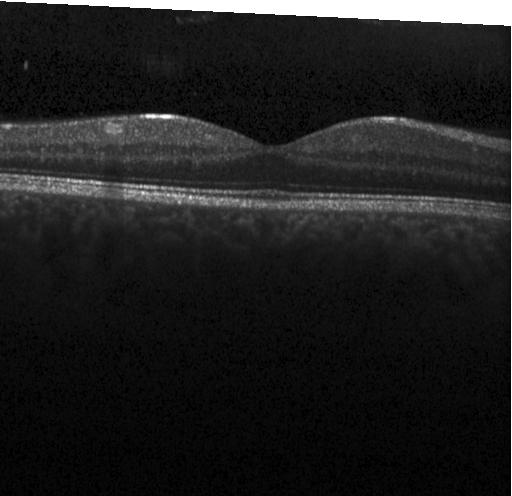
Heidelberg Spectralis, optical coherence tomography B-scan, spectral-domain optical coherence tomography — The scan shows no CNV, no DME, and no drusen.